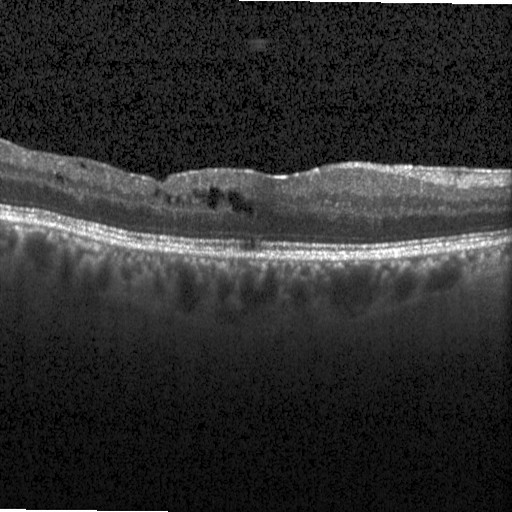

Retinal OCT B-scan, instrument: Heidelberg Spectralis, through the macula — Diabetic macular edema.